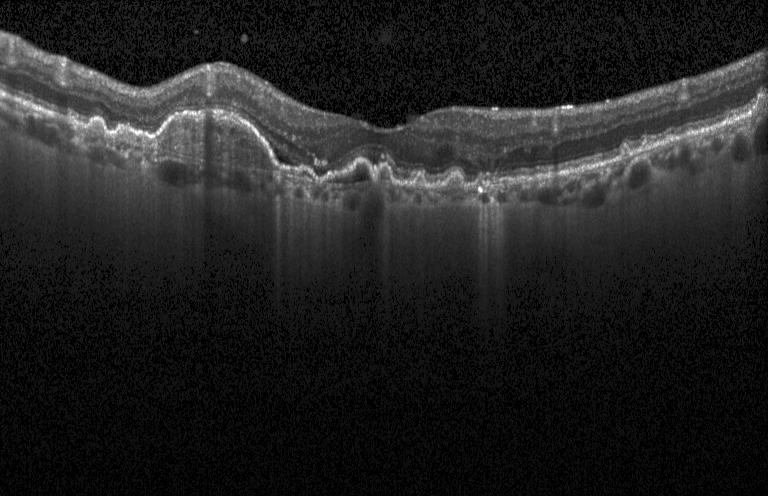
Optical coherence tomography B-scan.
Diagnosis: a choroidal neovascular membrane.